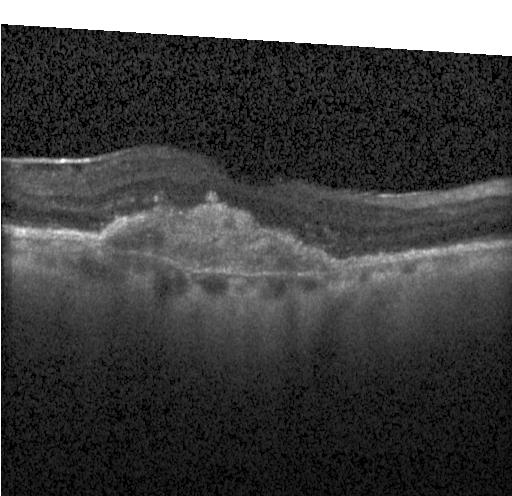 Dx: a choroidal neovascular membrane.